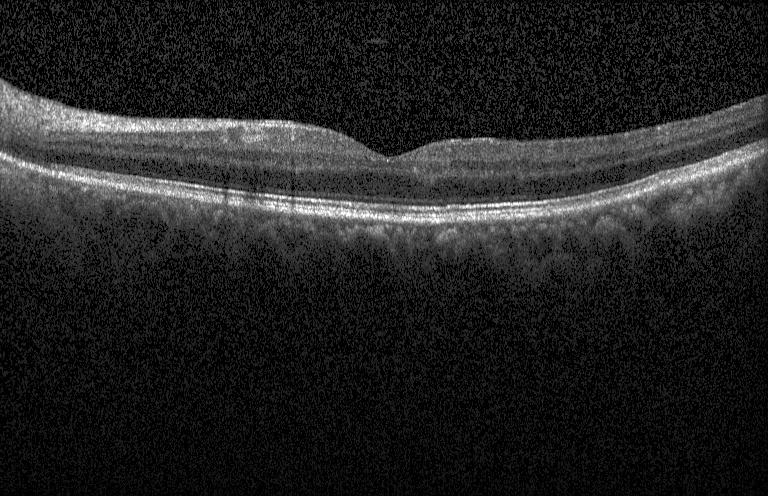

Heidelberg Spectralis OCT system, retinal OCT cross-section
Macular OCT: no choroidal neovascularization, diabetic macular edema, or drusen.